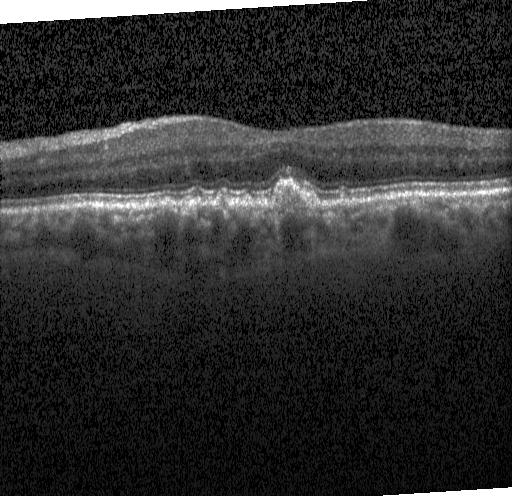
Dx: sub-RPE drusenoid deposits.